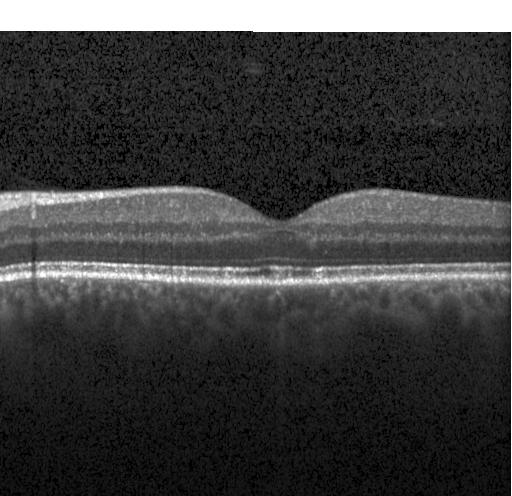

Spectral-domain OCT, OCT B-scan, acquired on a Heidelberg Spectralis.
Diagnosis: no CNV, DME, or drusen.